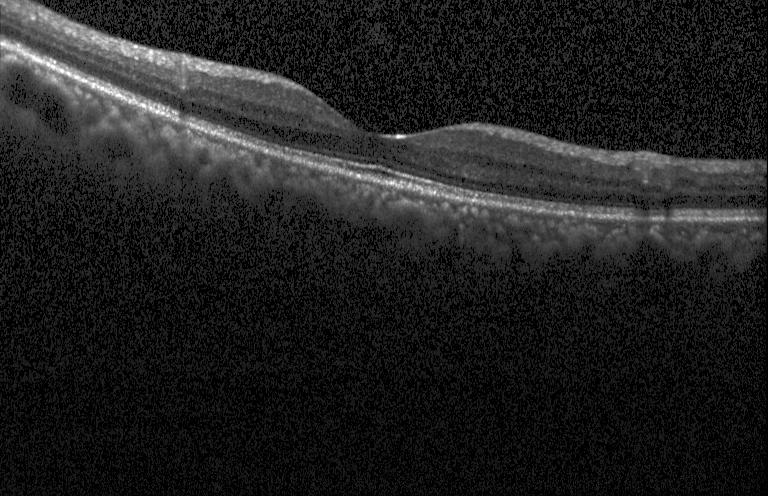

Heidelberg Spectralis OCT system, optical coherence tomography B-scan.
Impression: no choroidal neovascularization, diabetic macular edema, or drusen.